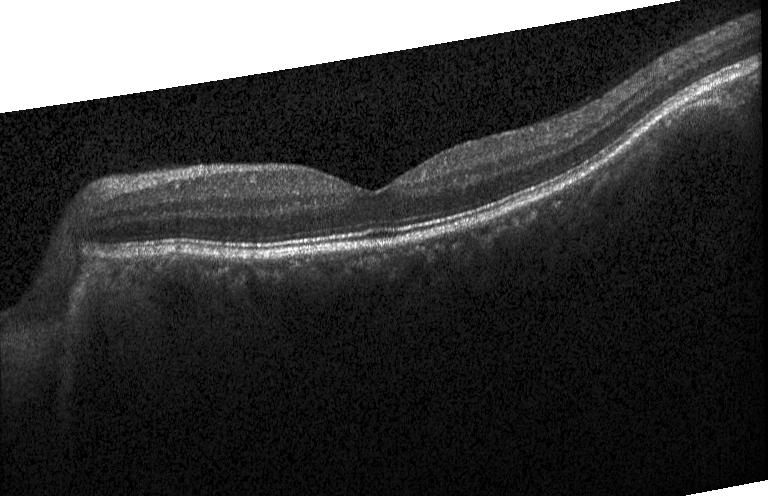

Spectral-domain optical coherence tomography, Heidelberg Spectralis OCT system, optical coherence tomography B-scan — Macular OCT: no choroidal neovascularization, diabetic macular edema, or drusen.